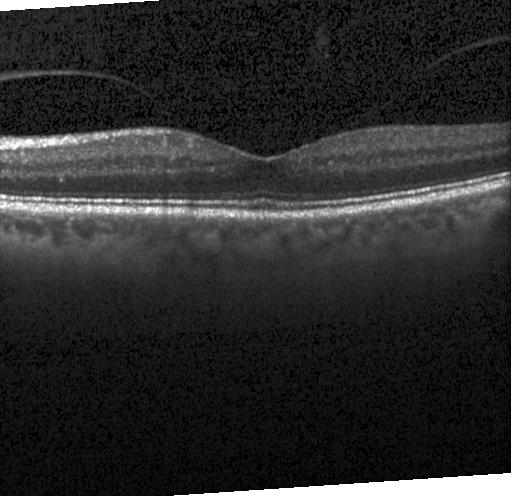

OCT B-scan; acquired on a Heidelberg Spectralis. OCT finding: no CNV, no DME, and no drusen.